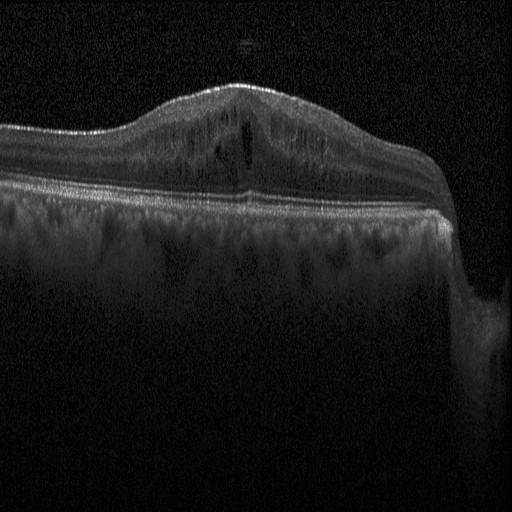 Retinal OCT cross-section, horizontal scan through the fovea, spectral-domain OCT. Assessment: diabetic macular edema (DME).